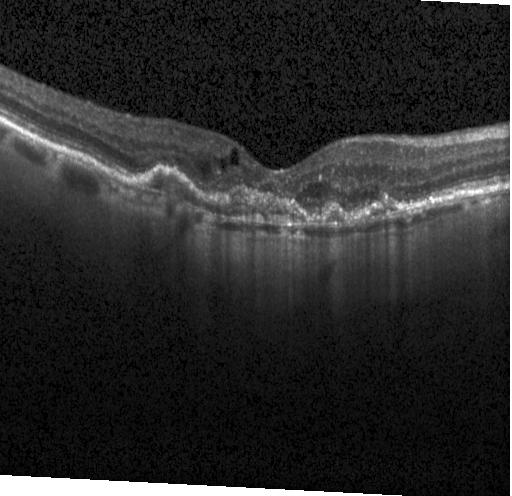 OCT line scan.
Assessment: a choroidal neovascular membrane.